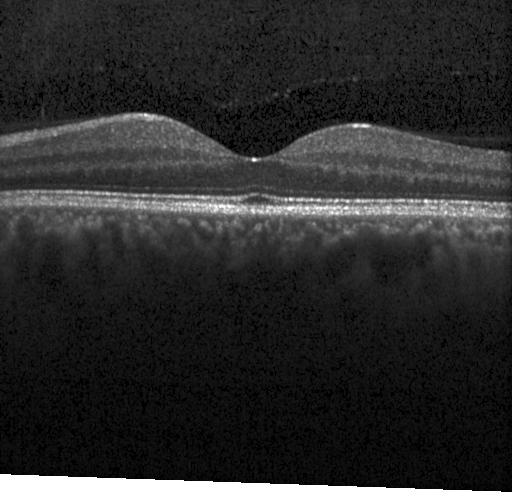 OCT line scan. Assessment: no choroidal neovascularization, diabetic macular edema, or drusen.